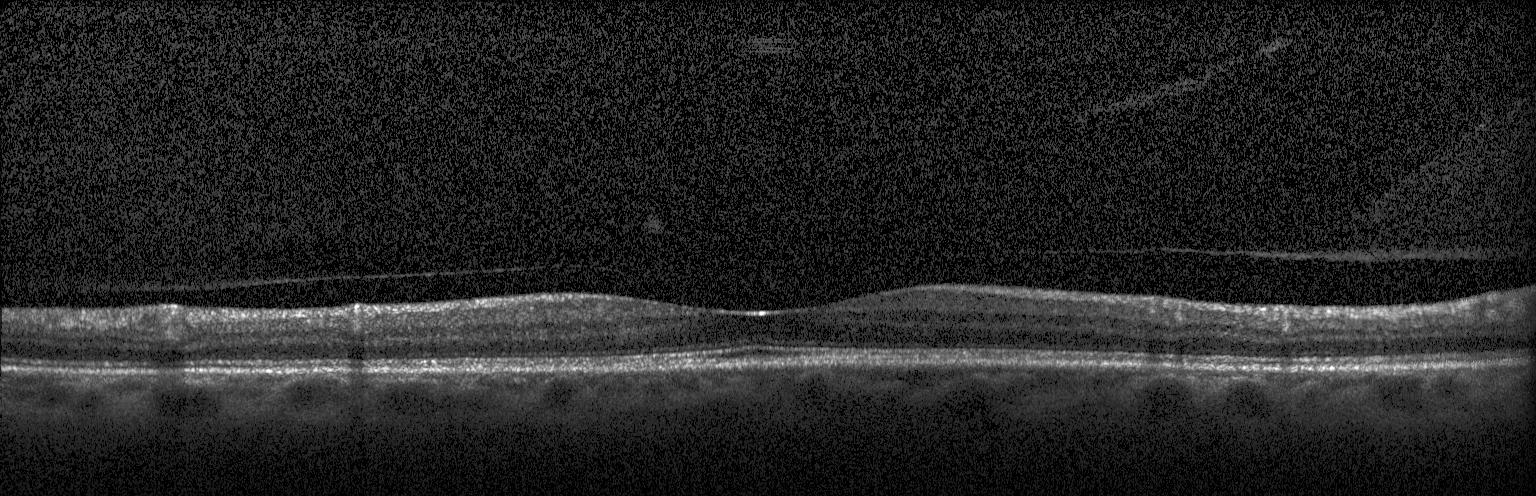

OCT B-scan
Finding: neither CNV, DME, nor drusen.